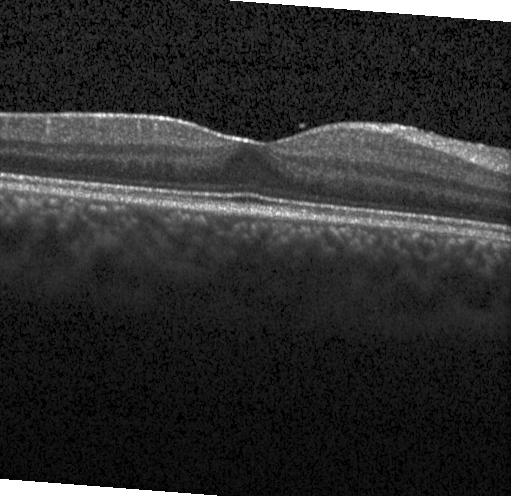
Acquired on a Heidelberg Spectralis · horizontal scan through the fovea · optical coherence tomography scan. OCT finding: no choroidal neovascularization, no diabetic macular edema, and no drusen.